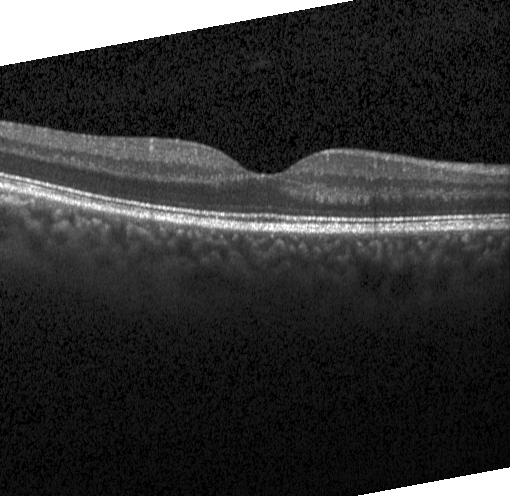
Impression: no choroidal neovascularization, no diabetic macular edema, and no drusen.